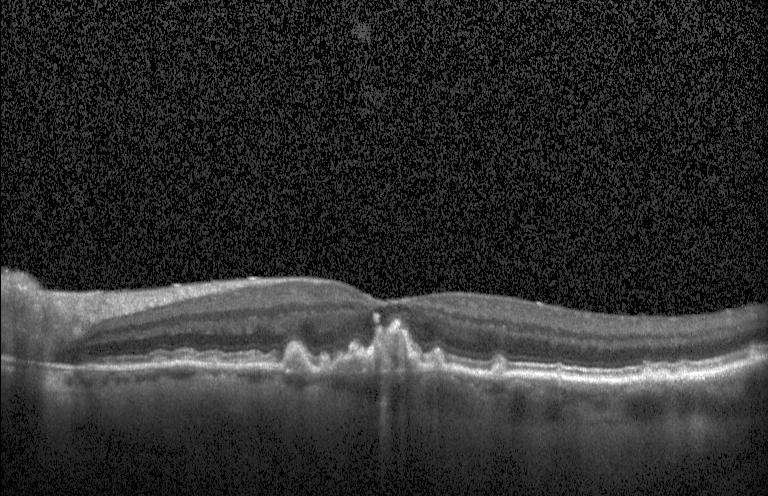

Dx: a choroidal neovascular membrane.